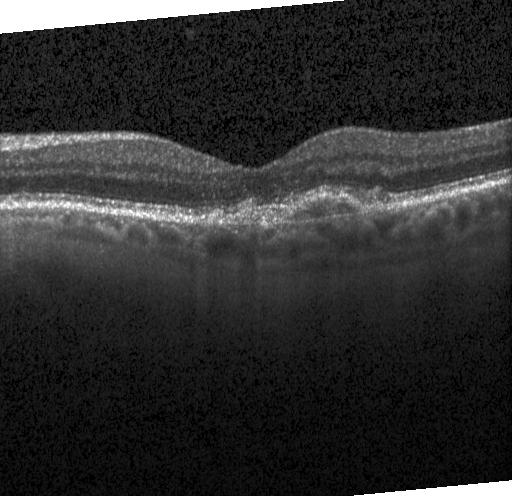 A choroidal neovascular membrane.